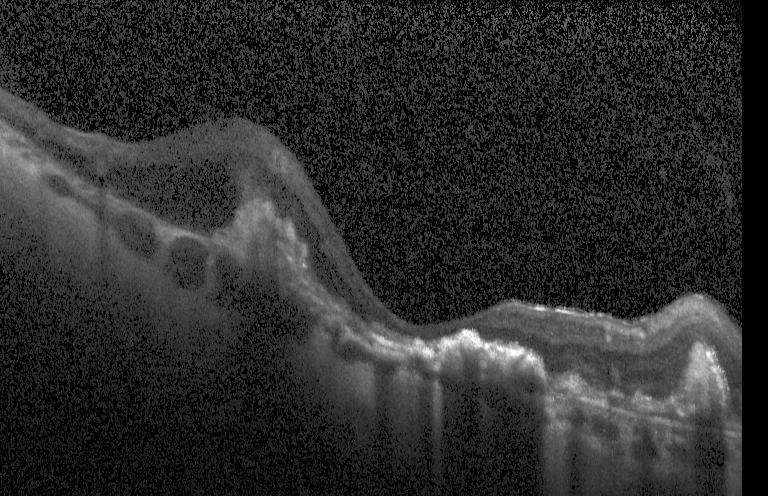

SD-OCT · horizontal scan through the fovea · OCT B-scan — The scan shows choroidal neovascularization (CNV).